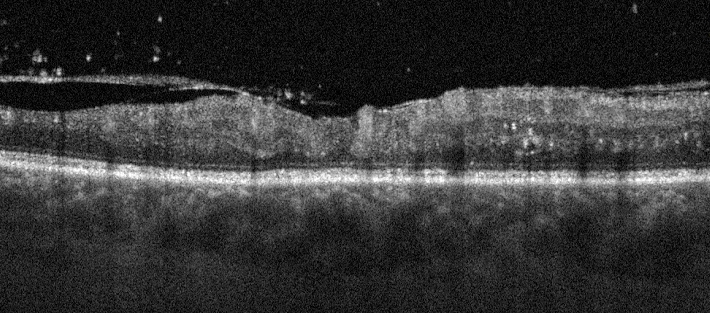
OCT line scan, through the macula.
Dx: diabetic macular edema.